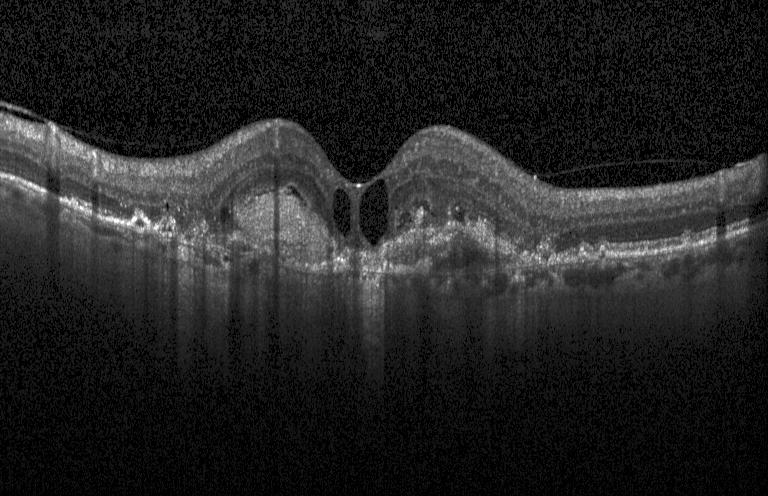
Horizontal scan through the fovea. Spectral-domain optical coherence tomography. OCT B-scan — Impression: choroidal neovascularization.